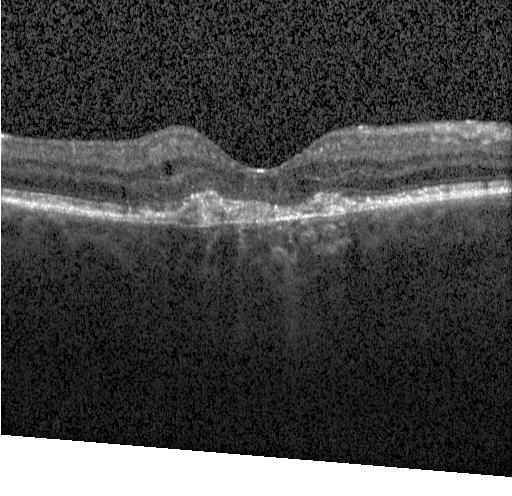

Dx: choroidal neovascularization (CNV).